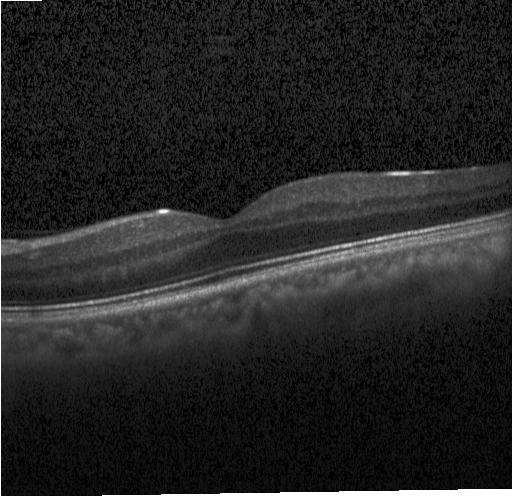 Macular scan, spectral-domain OCT, optical coherence tomography B-scan. The scan shows no choroidal neovascularization, no diabetic macular edema, and no drusen.